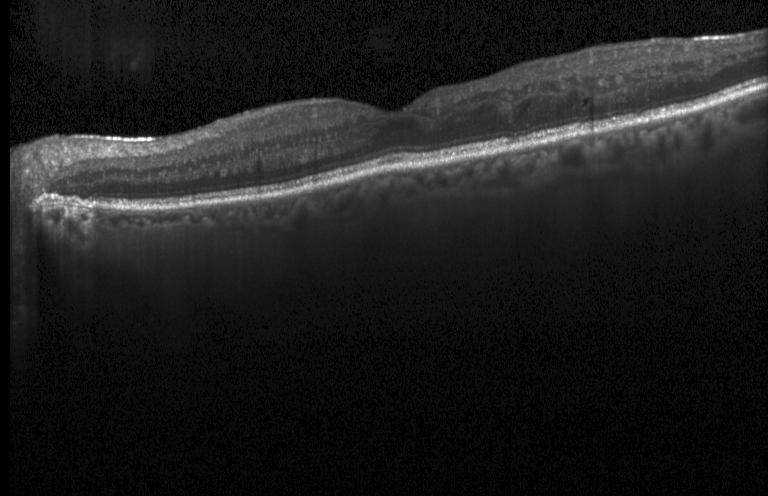 Finding: no evidence of choroidal neovascularization, diabetic macular edema, or drusen.